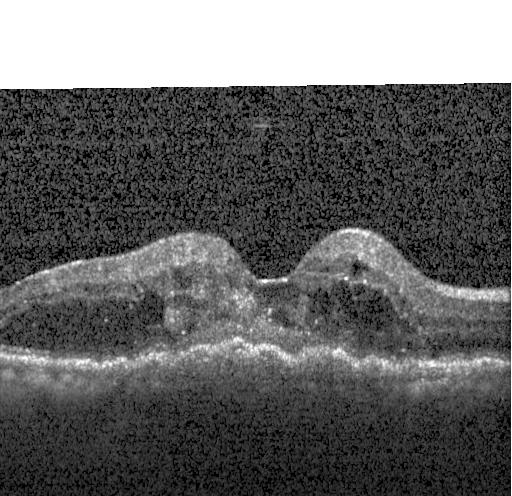 Through the macula, OCT B-scan, Heidelberg Spectralis, spectral-domain optical coherence tomography.
Impression: choroidal neovascularization (CNV).